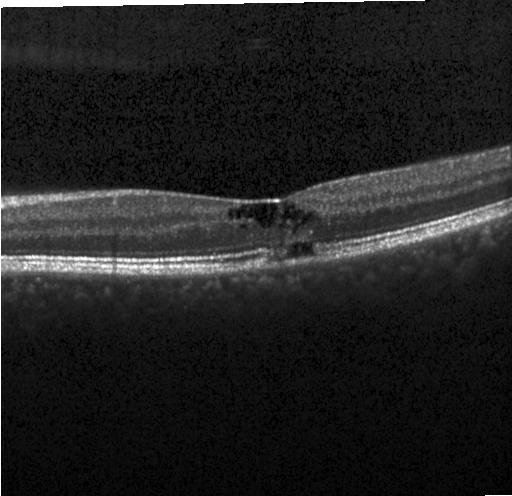
OCT line scan; spectral-domain optical coherence tomography — Impression: diabetic macular edema (DME).